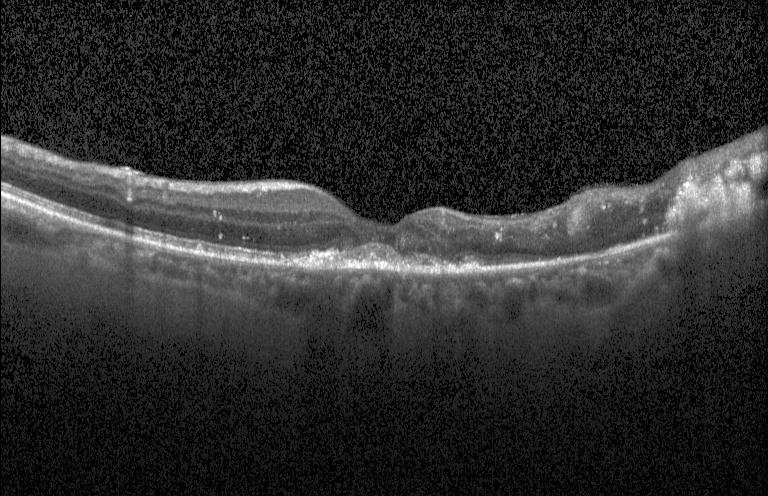
Heidelberg Spectralis OCT system · optical coherence tomography B-scan — Dx: CNV.